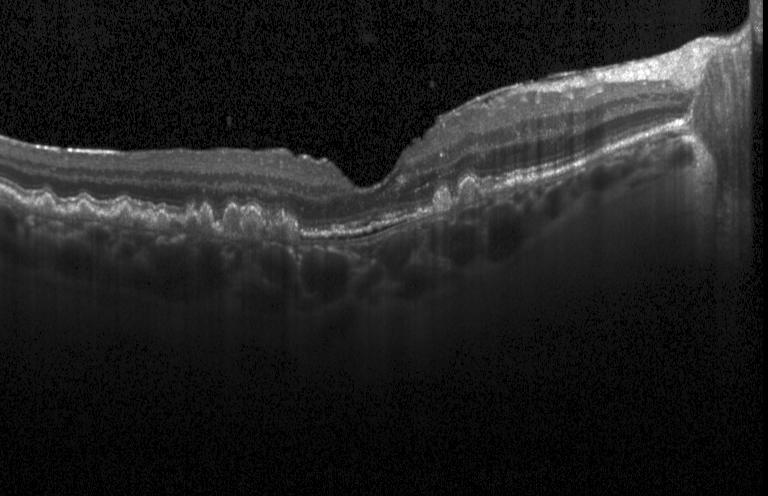
SD-OCT. OCT B-scan — Dx: a choroidal neovascular membrane.